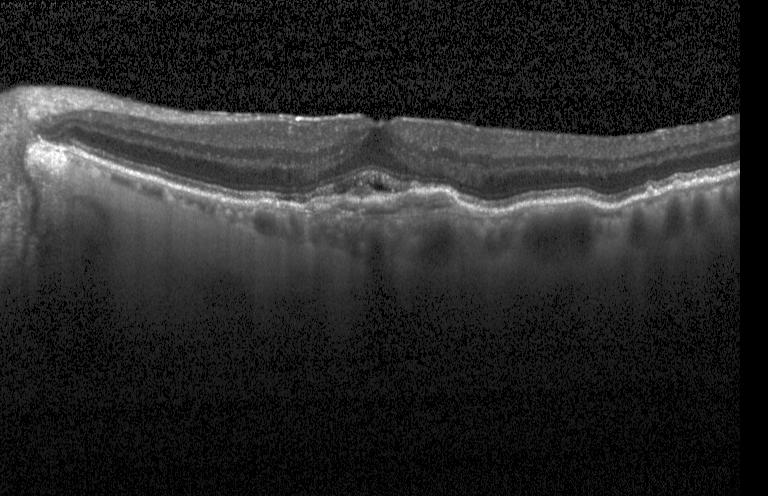

Through the macula. Instrument: Heidelberg Spectralis. SD-OCT. Optical coherence tomography scan. The scan shows a choroidal neovascular membrane.